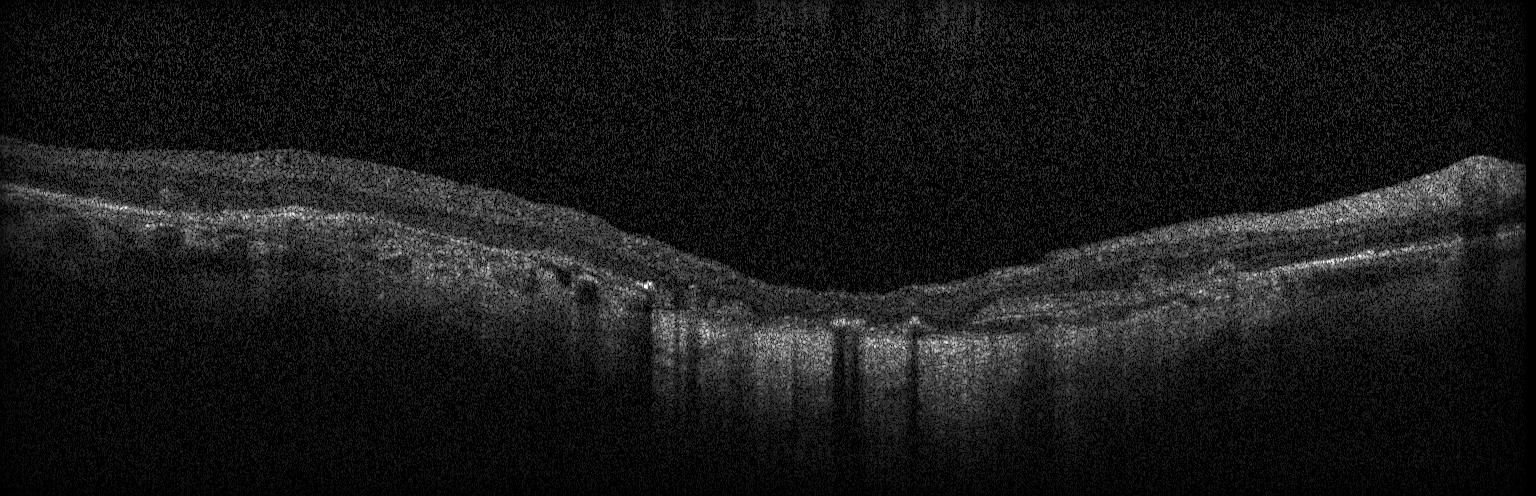 Centered on the fovea, retinal OCT B-scan, Heidelberg Spectralis, spectral-domain OCT.
Choroidal neovascularization (CNV).